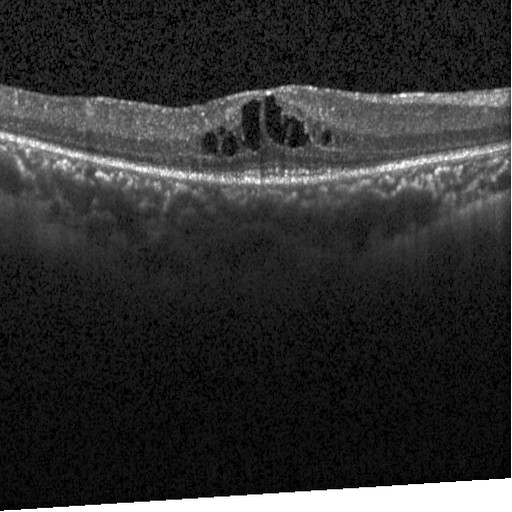 Horizontal scan through the fovea, OCT line scan, spectral-domain optical coherence tomography — OCT finding: diabetic macular edema.